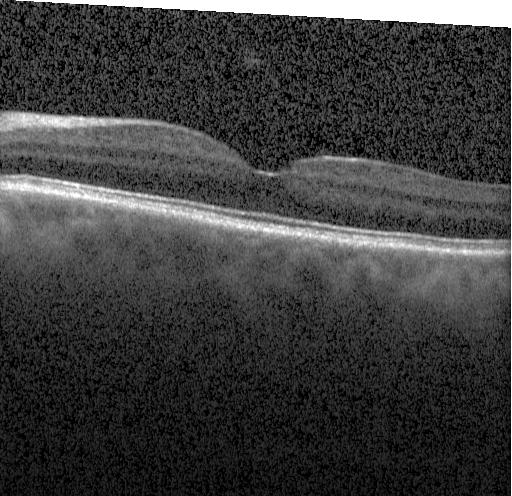

Spectral-domain OCT. Optical coherence tomography B-scan. Horizontal scan through the fovea.
Neither choroidal neovascularization, diabetic macular edema, nor drusen.